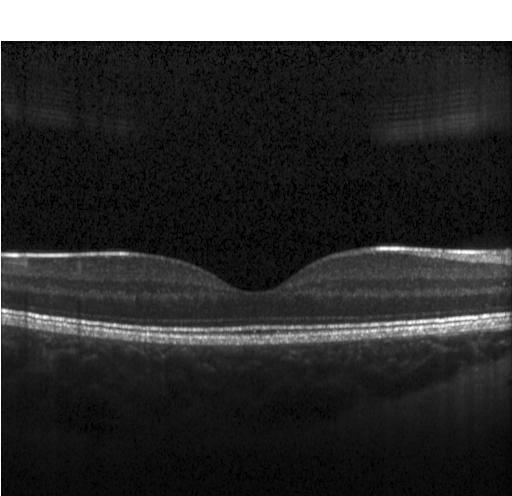
OCT B-scan
OCT finding: no CNV, DME, or drusen.